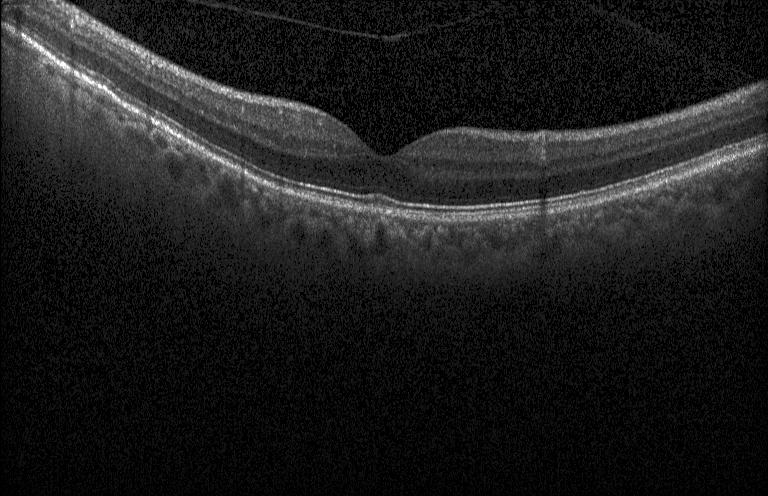 Instrument: Heidelberg Spectralis · spectral-domain OCT · horizontal scan through the fovea · optical coherence tomography scan — Finding: no choroidal neovascularization, diabetic macular edema, or drusen.